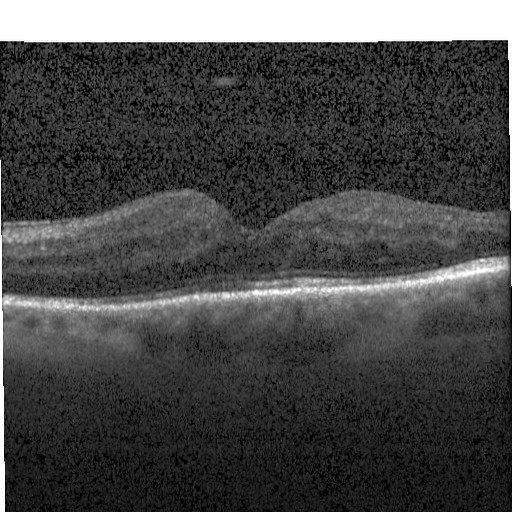

Macular OCT demonstrating diabetic macular edema (DME).